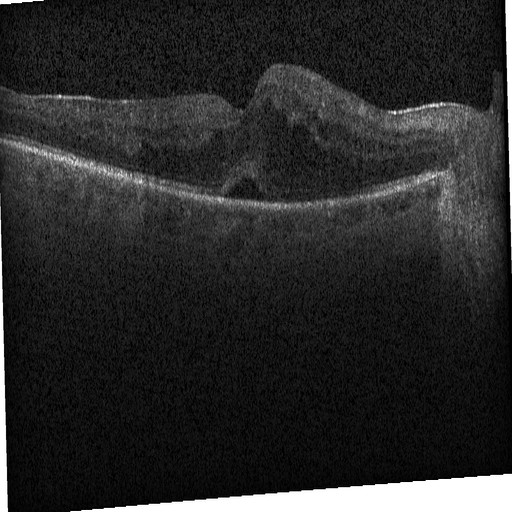
Dx: diabetic macular edema.